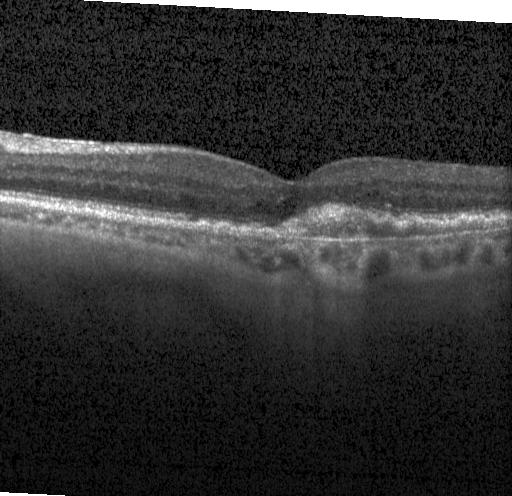 OCT scan showing a choroidal neovascular membrane.